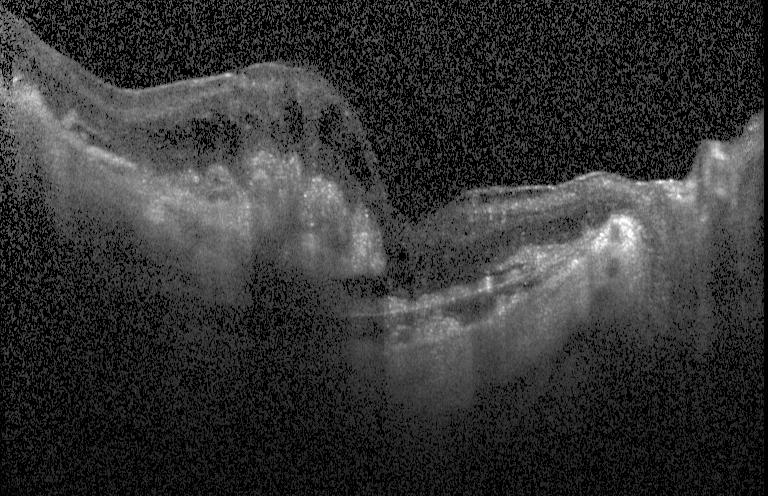 Finding: CNV.